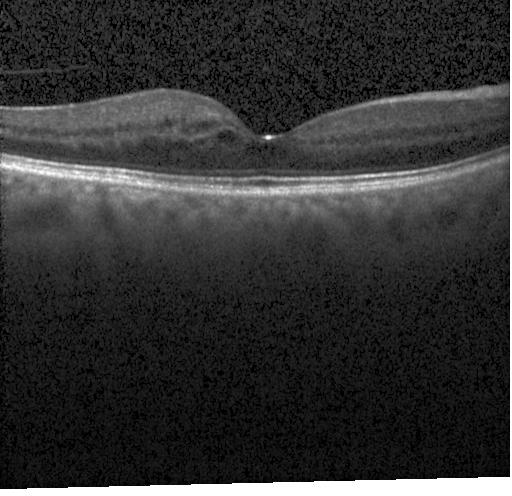

Spectral-domain optical coherence tomography; fovea-centered; instrument: Heidelberg Spectralis; retinal OCT cross-section
Diagnosis: DME.